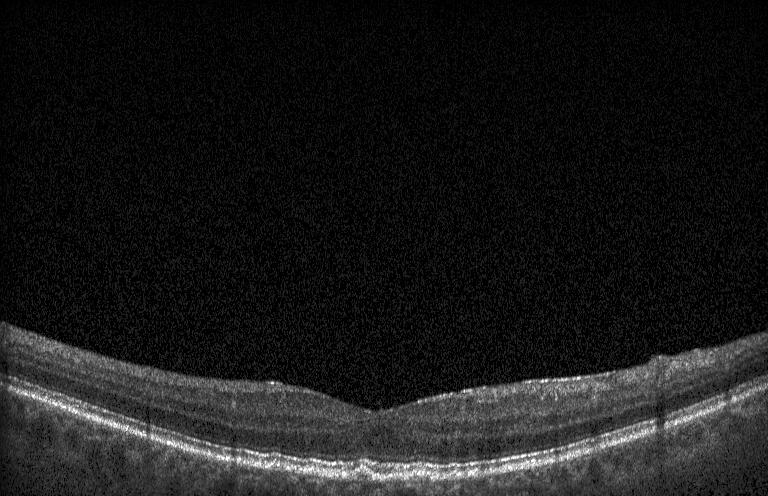
Macular scan · SD-OCT · OCT B-scan · Heidelberg Spectralis OCT system
Impression: drusen.